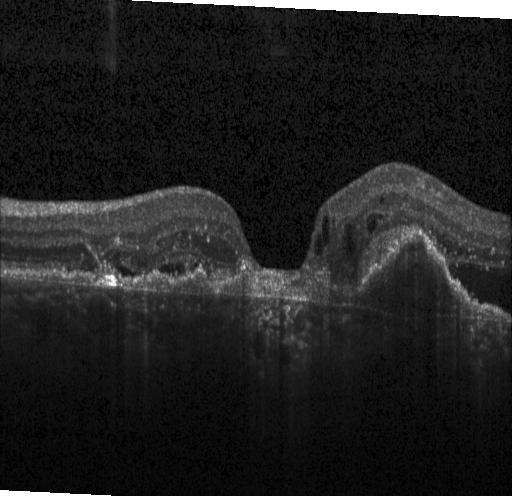 Heidelberg Spectralis OCT system, spectral-domain optical coherence tomography, retinal OCT B-scan.
Finding: choroidal neovascularization.